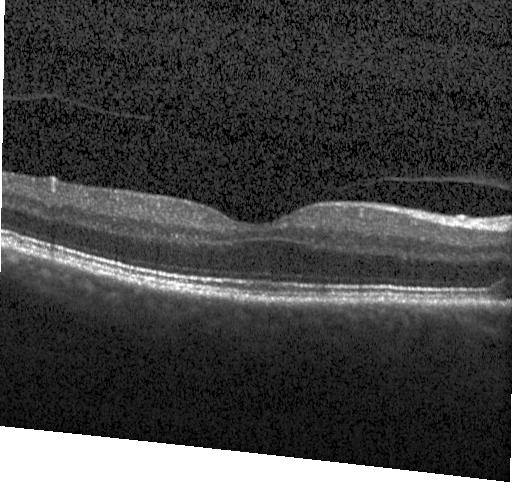 Horizontal scan through the fovea · optical coherence tomography scan.
Finding: no evidence of choroidal neovascularization, diabetic macular edema, or drusen.